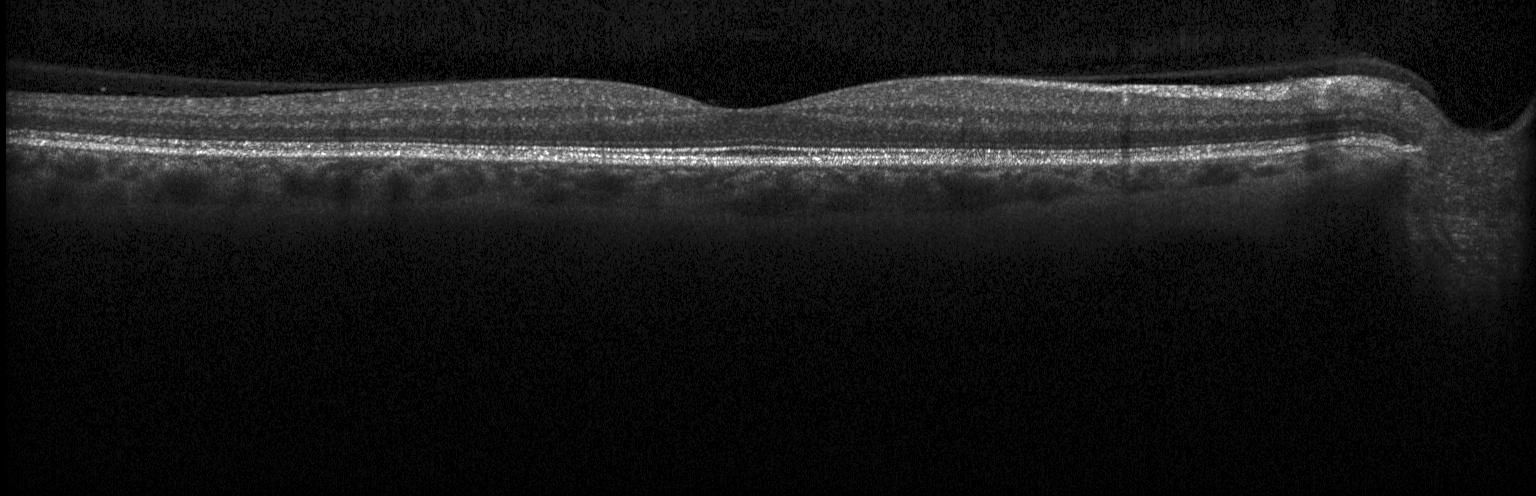 Retinal OCT cross-section
Diagnosis: no CNV, no DME, and no drusen.